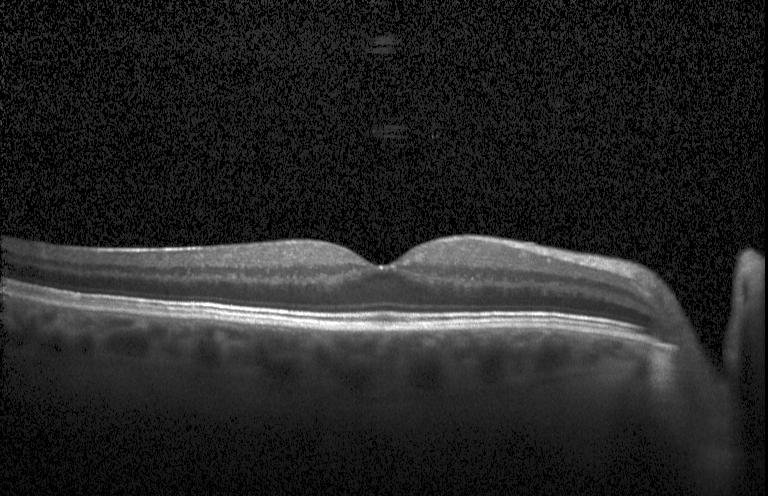 Spectral-domain OCT. Heidelberg Spectralis OCT system. Retinal OCT B-scan — Finding: neither CNV, DME, nor drusen.